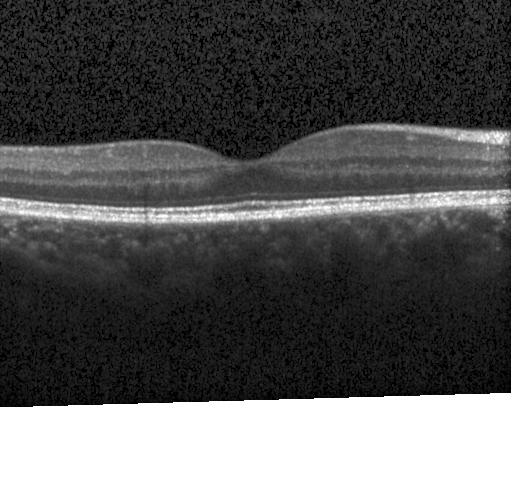

Assessment: no CNV, DME, or drusen.